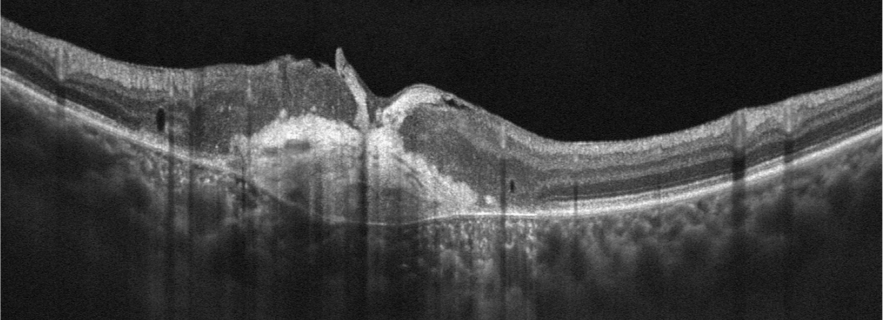 OCT finding: AMD.